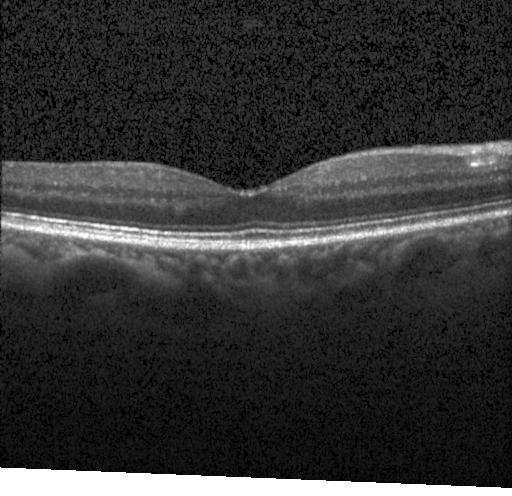
Optical coherence tomography B-scan. Impression: no evidence of choroidal neovascularization, diabetic macular edema, or drusen.